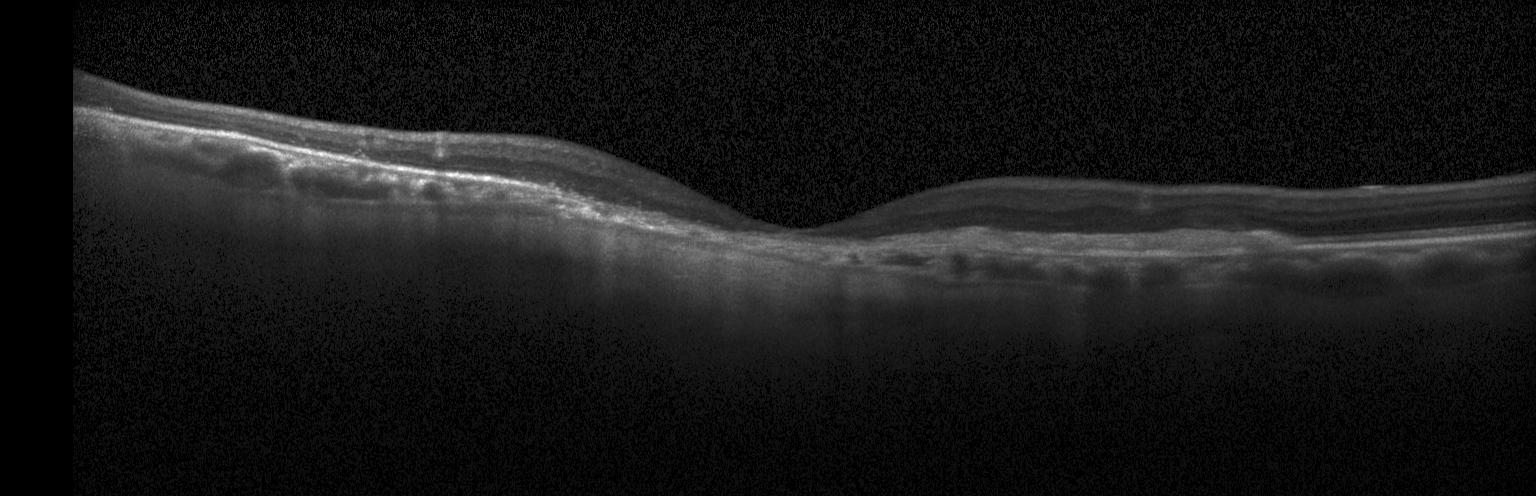

Instrument: Heidelberg Spectralis, OCT line scan, macular scan. Diagnosis: a choroidal neovascular membrane.